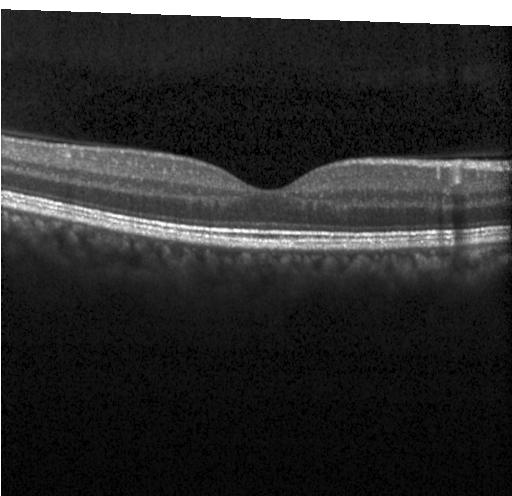

Assessment: no evidence of choroidal neovascularization, diabetic macular edema, or drusen.